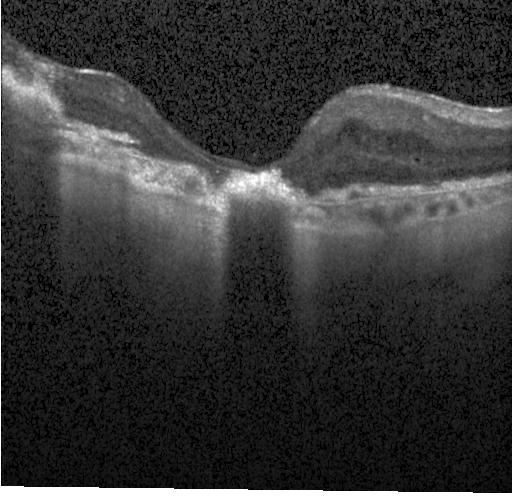

Retinal OCT cross-section — This B-scan demonstrates CNV.